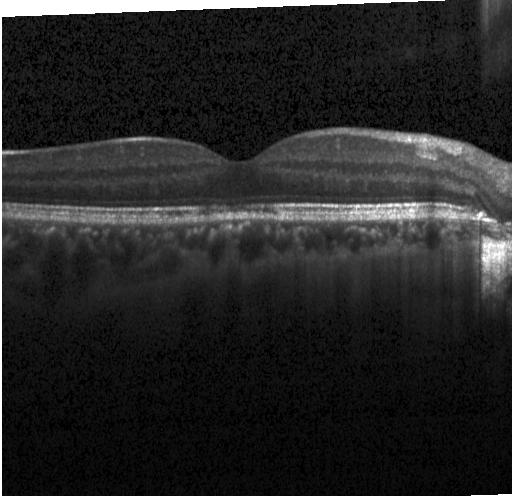

Impression: neither choroidal neovascularization, diabetic macular edema, nor drusen.